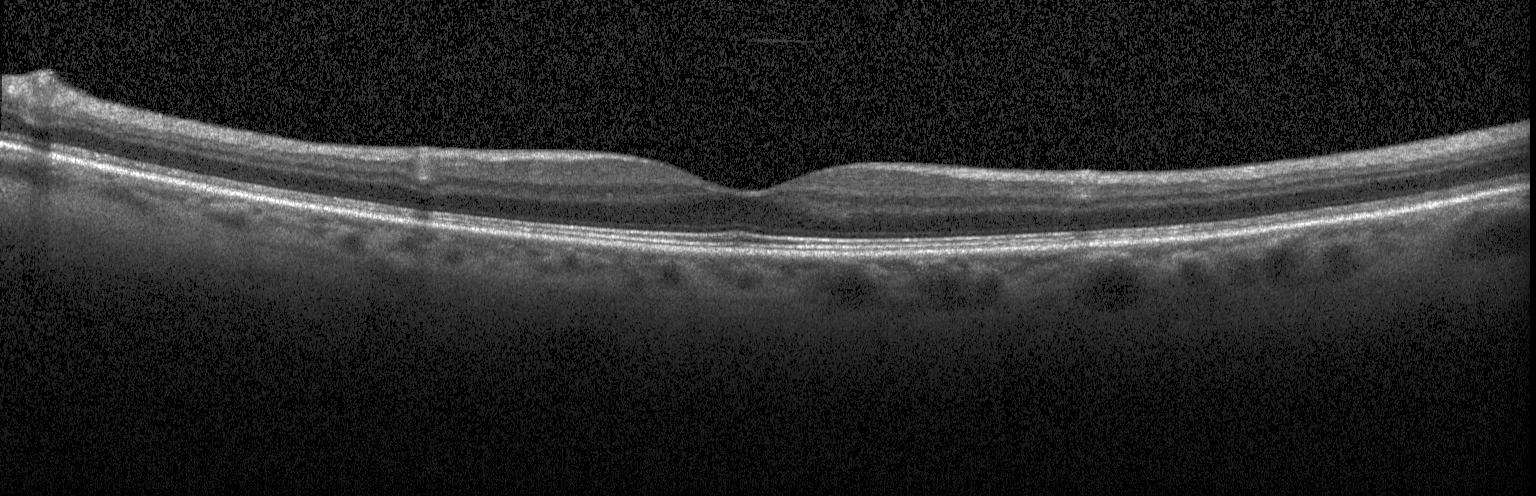
Acquired on a Heidelberg Spectralis, through the macula, OCT line scan, spectral-domain optical coherence tomography — Macular OCT: neither choroidal neovascularization, diabetic macular edema, nor drusen.